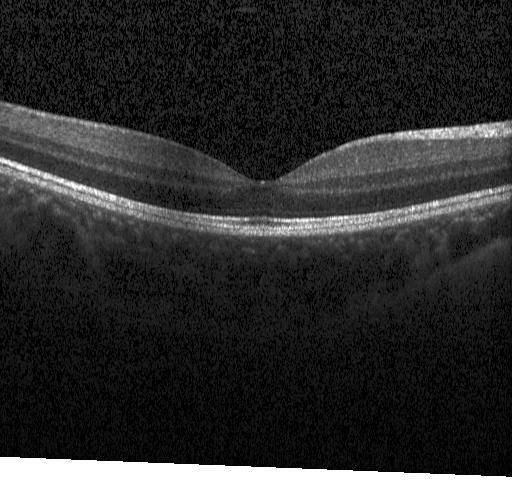 No CNV, DME, or drusen.